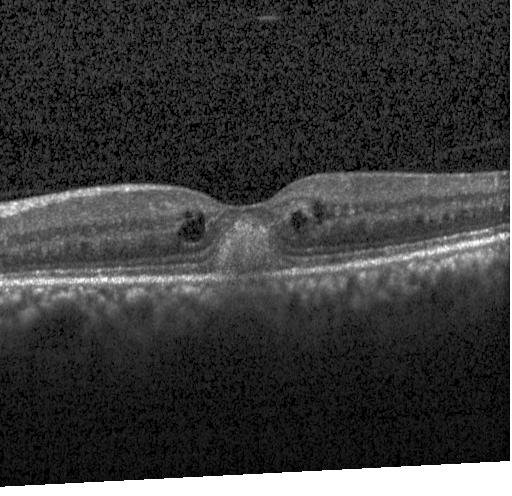 OCT B-scan. Fovea-centered. Impression: choroidal neovascularization.